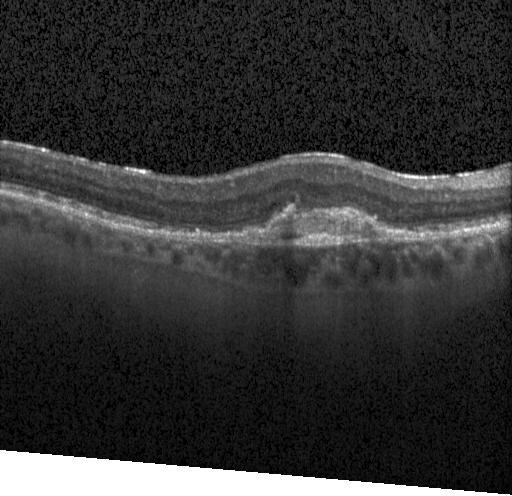

Spectral-domain OCT B-scan: a choroidal neovascular membrane.